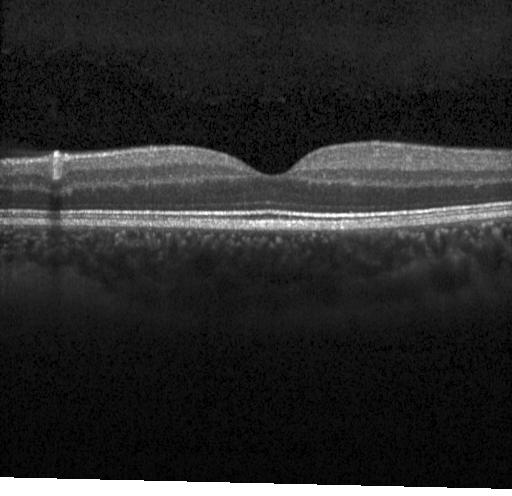

Optical coherence tomography scan.
Diagnosis: no choroidal neovascularization, no diabetic macular edema, and no drusen.